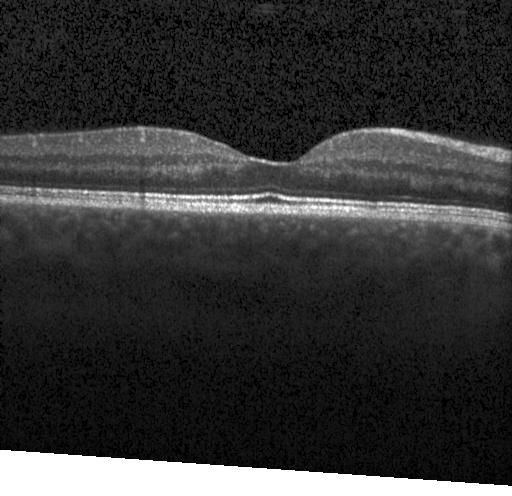
Retinal OCT B-scan — No choroidal neovascularization, no diabetic macular edema, and no drusen.